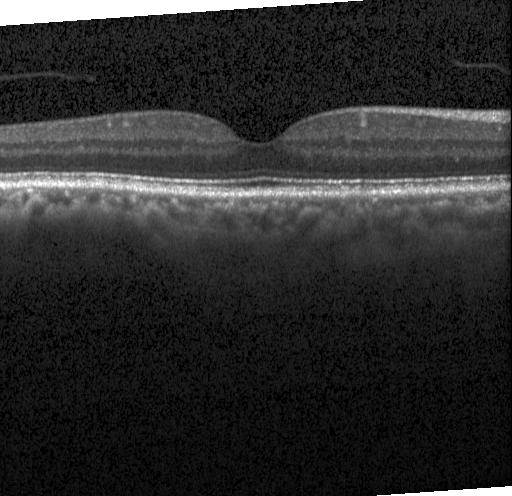 Heidelberg Spectralis OCT system; centered on the fovea; optical coherence tomography B-scan.
Finding: no evidence of choroidal neovascularization, diabetic macular edema, or drusen.